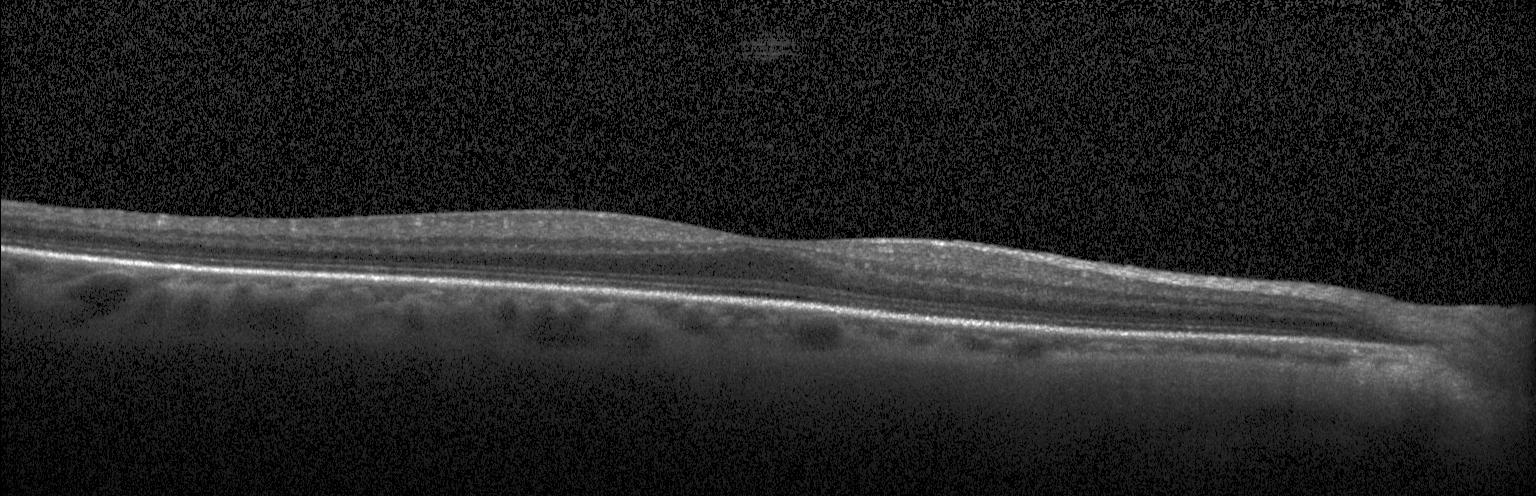 Optical coherence tomography B-scan.
Macular OCT: no CNV, DME, or drusen.